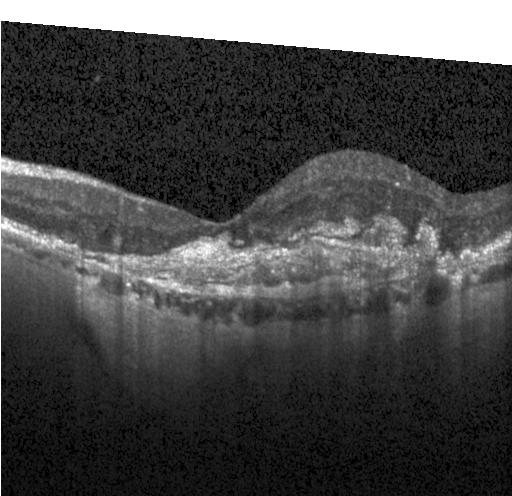
Impression: a choroidal neovascular membrane.